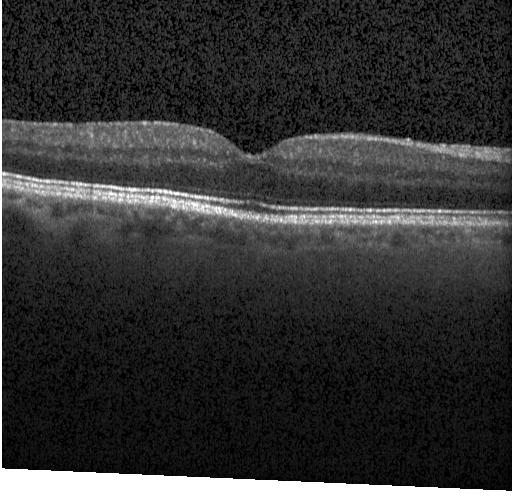
Heidelberg Spectralis OCT system, optical coherence tomography scan, spectral-domain OCT
No evidence of CNV, DME, or drusen.